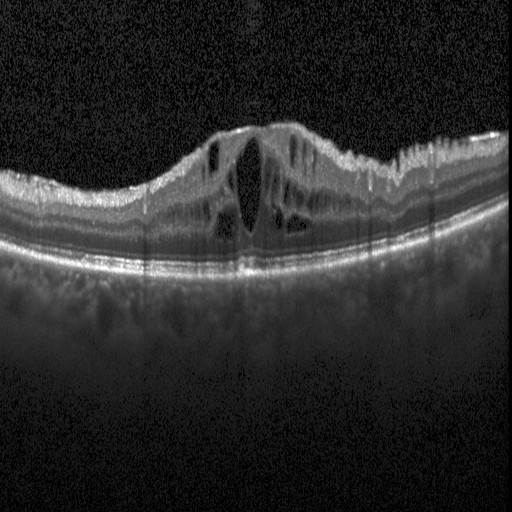
Diagnosis: DME.